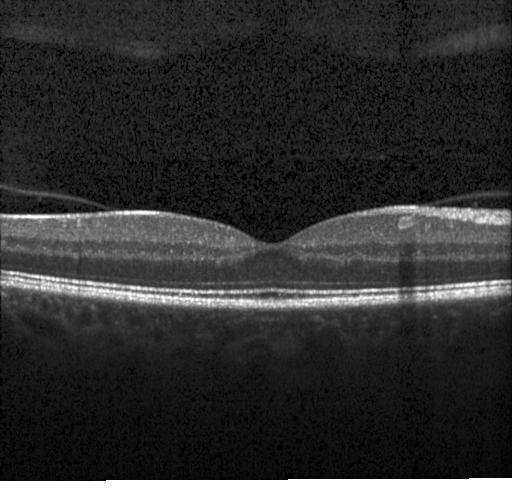 Macular OCT: no CNV, DME, or drusen.